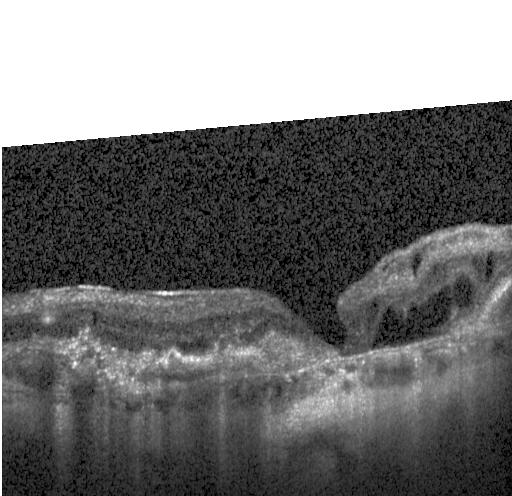
Retinal OCT cross-section — Diagnosis: choroidal neovascularization.